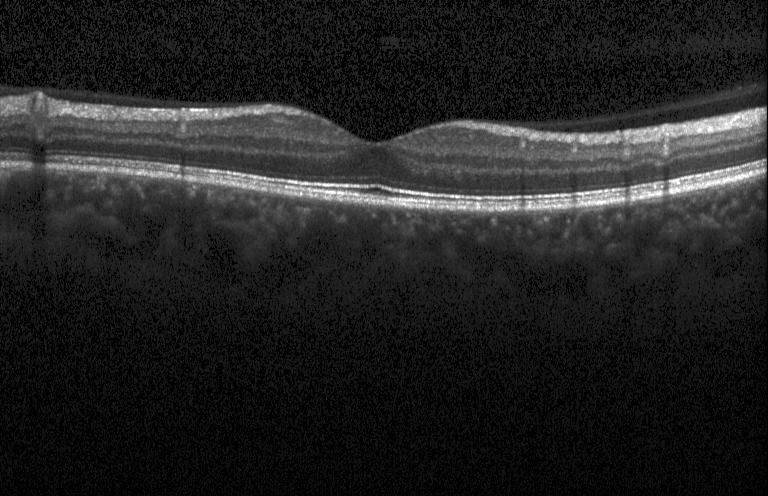
This B-scan demonstrates no evidence of choroidal neovascularization, diabetic macular edema, or drusen.